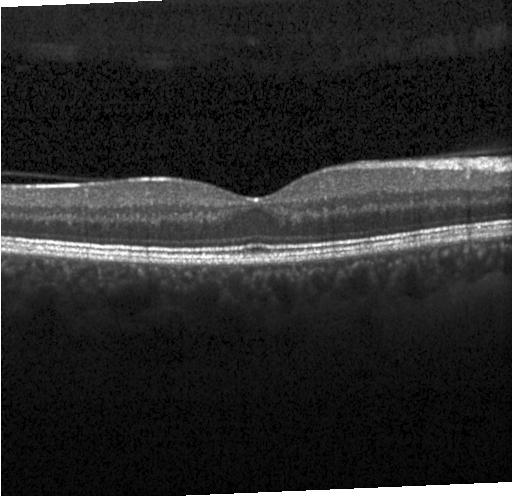 OCT line scan
Assessment: no choroidal neovascularization, no diabetic macular edema, and no drusen.